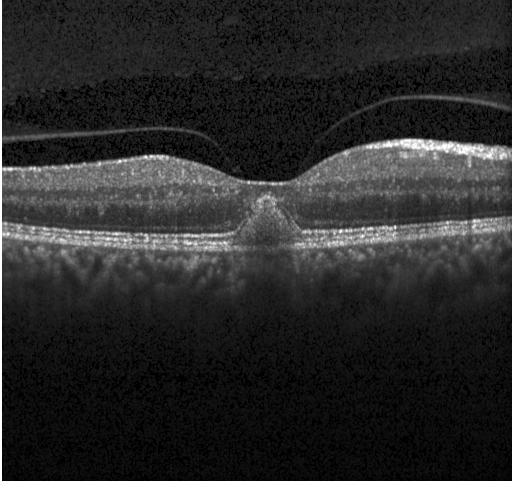

Finding: choroidal neovascularization.